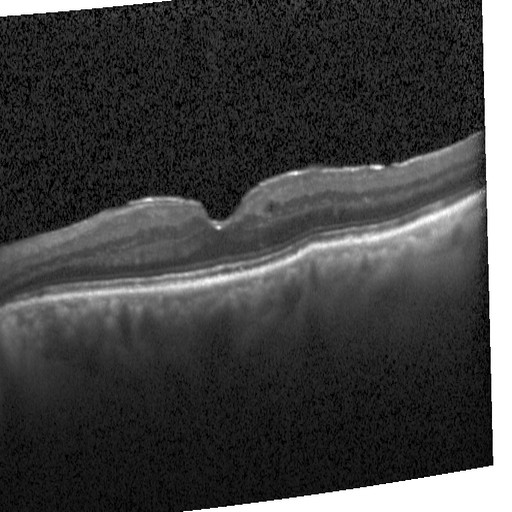

Heidelberg Spectralis. Retinal OCT cross-section. Spectral-domain optical coherence tomography — Impression: diabetic macular edema (DME).